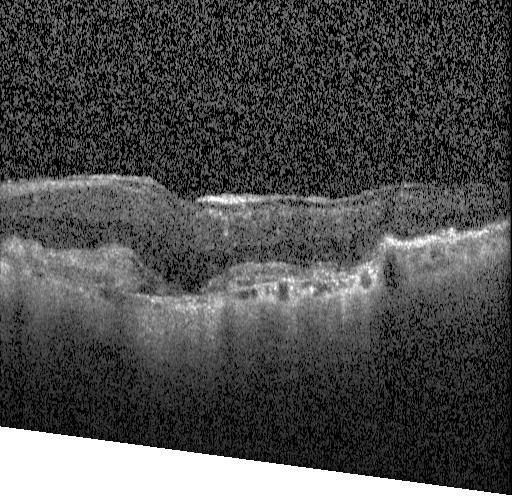 OCT finding: a choroidal neovascular membrane.